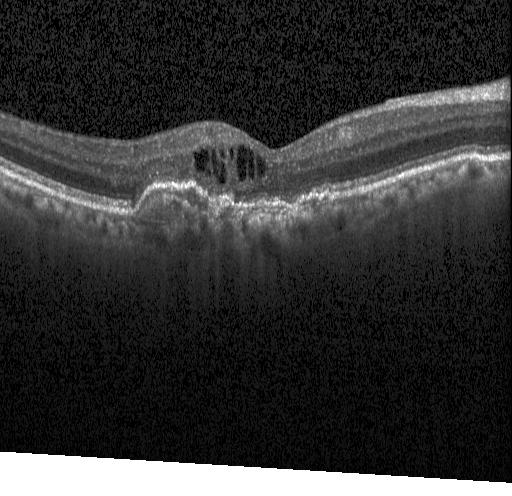

SD-OCT. Optical coherence tomography scan. Fovea-centered. Heidelberg Spectralis OCT system.
Finding: a choroidal neovascular membrane.